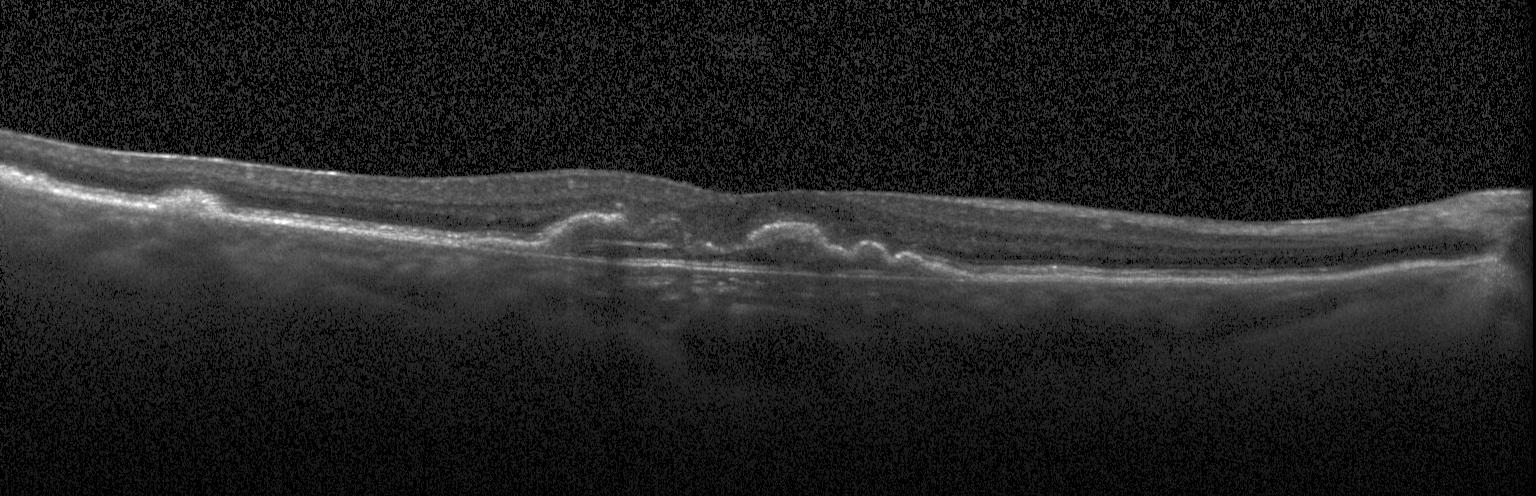

OCT scan showing CNV.